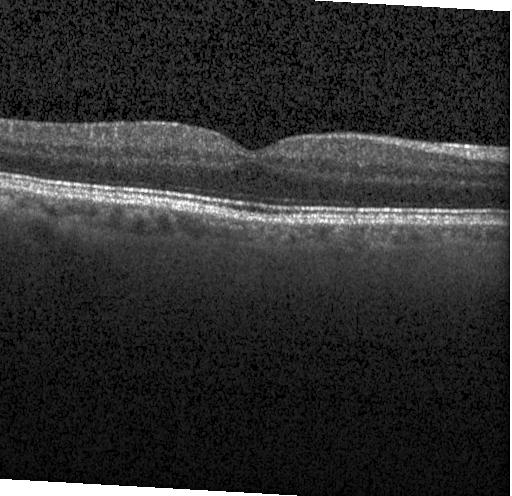 Impression: no evidence of choroidal neovascularization, diabetic macular edema, or drusen.